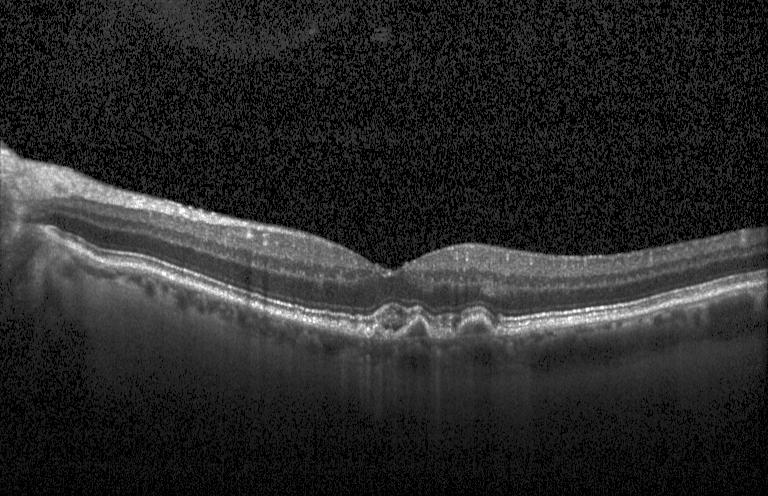
OCT B-scan.
Impression: a choroidal neovascular membrane.